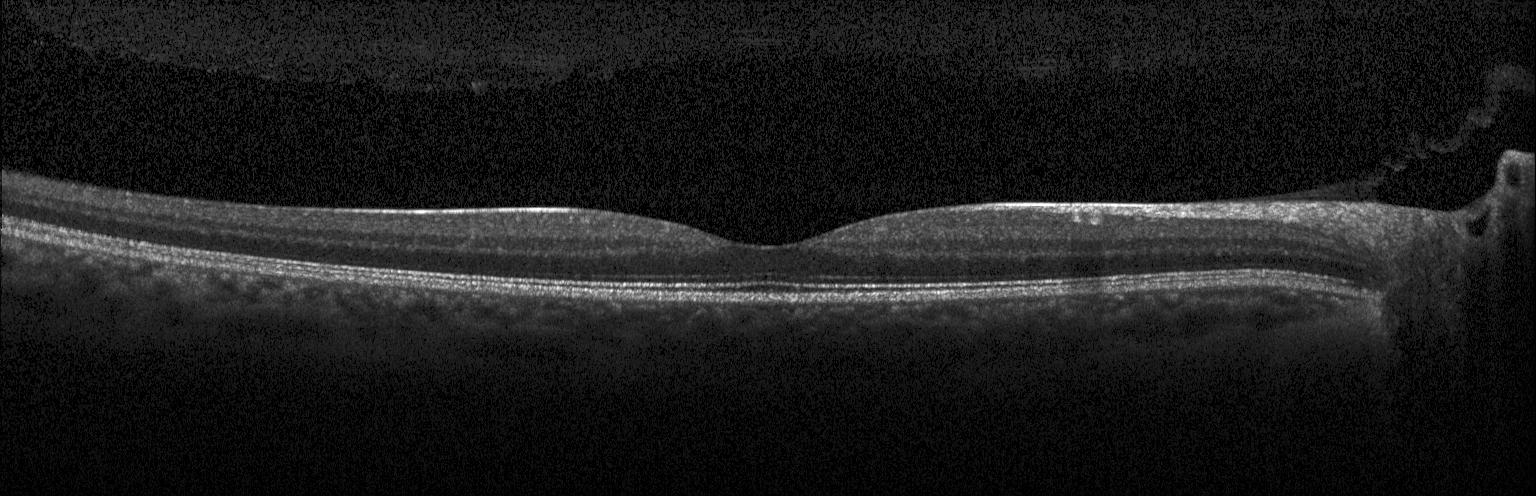

Instrument: Heidelberg Spectralis, retinal OCT B-scan, spectral-domain OCT. This B-scan demonstrates no choroidal neovascularization, no diabetic macular edema, and no drusen.